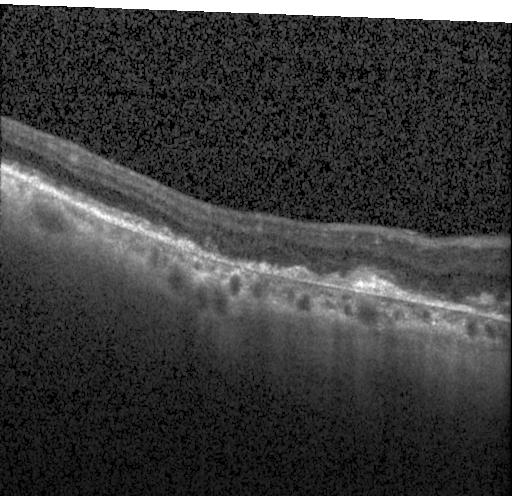 Impression: choroidal neovascularization.